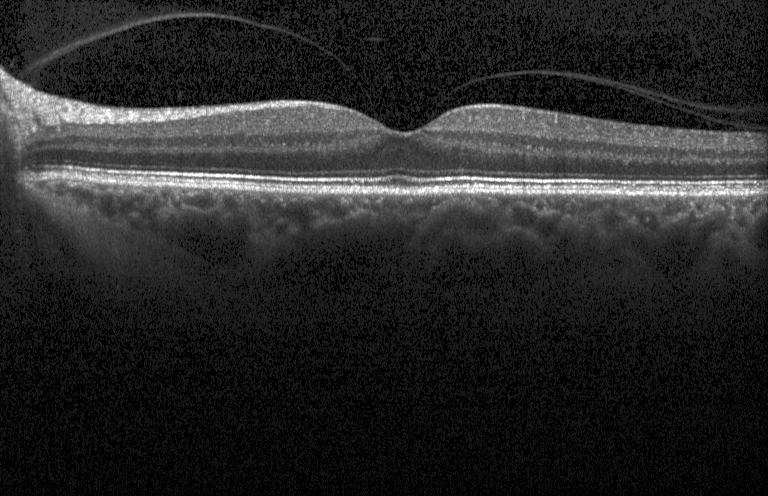

Retinal OCT cross-section showing no CNV, no DME, and no drusen.